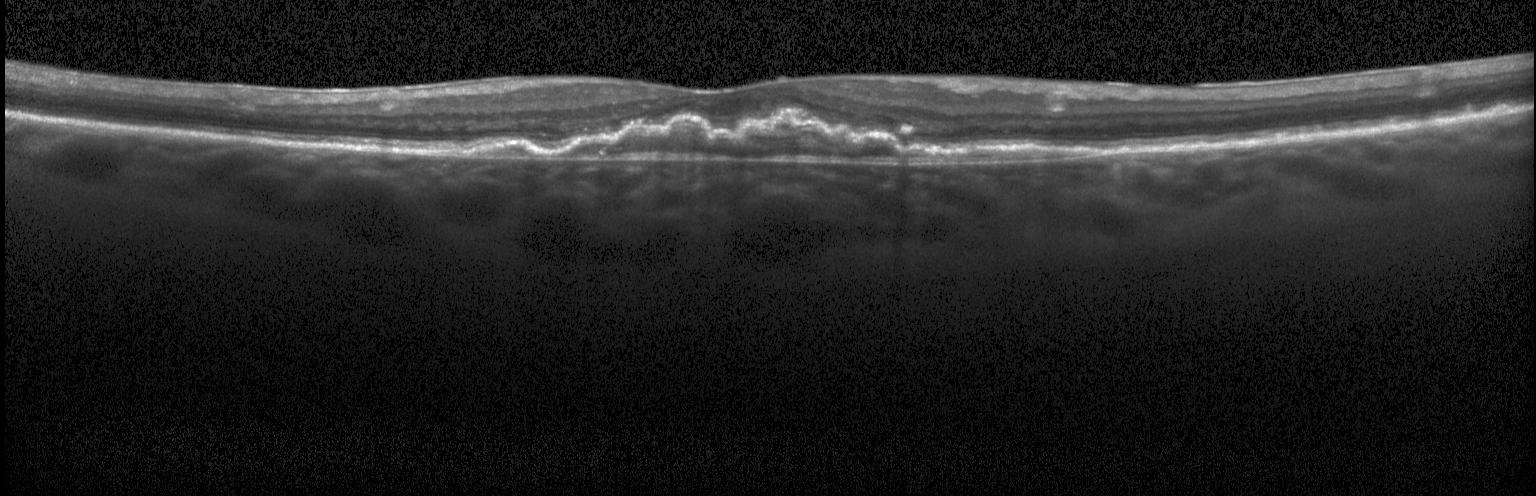
Optical coherence tomography scan.
Diagnosis: a choroidal neovascular membrane.